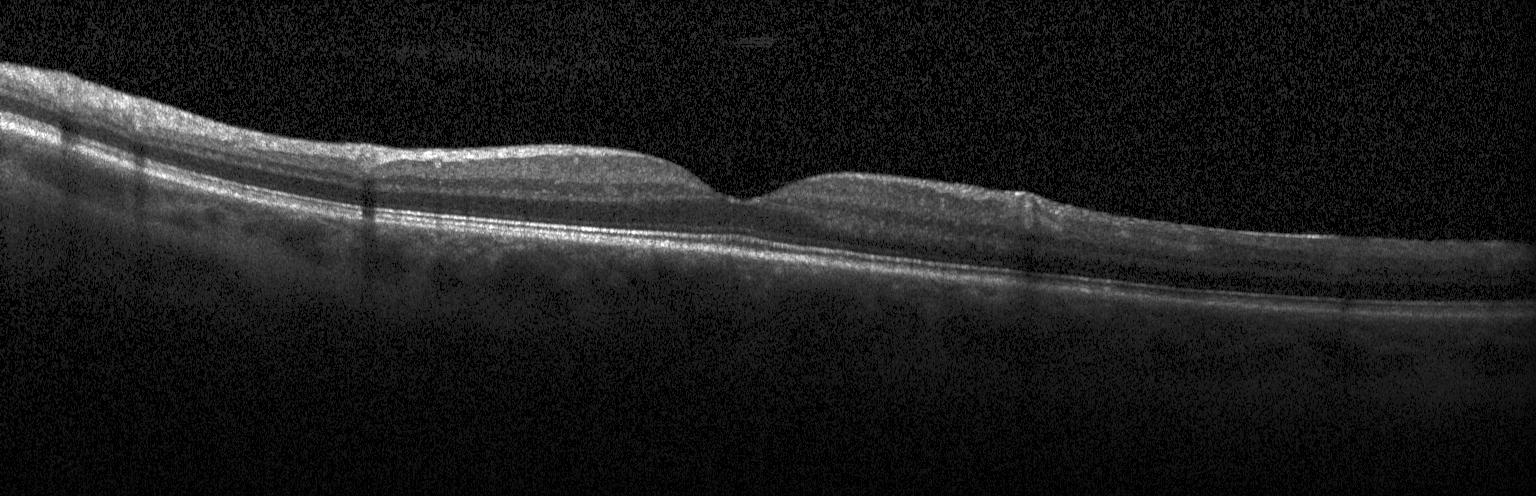 Fovea-centered; optical coherence tomography B-scan. Assessment: no evidence of CNV, DME, or drusen.